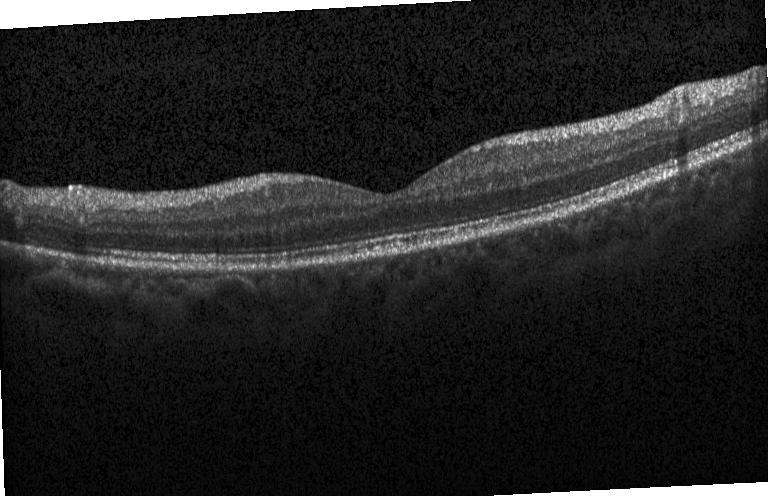
Spectral-domain optical coherence tomography. Instrument: Heidelberg Spectralis. Horizontal scan through the fovea. Retinal OCT cross-section — No CNV, DME, or drusen.